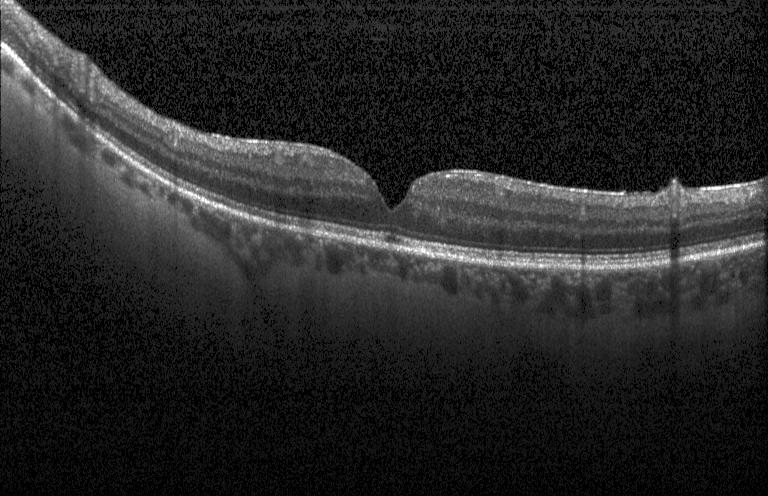

Assessment: neither choroidal neovascularization, diabetic macular edema, nor drusen.